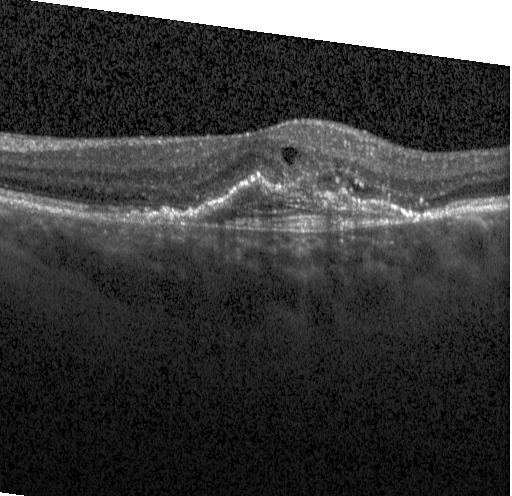

Impression: a choroidal neovascular membrane.